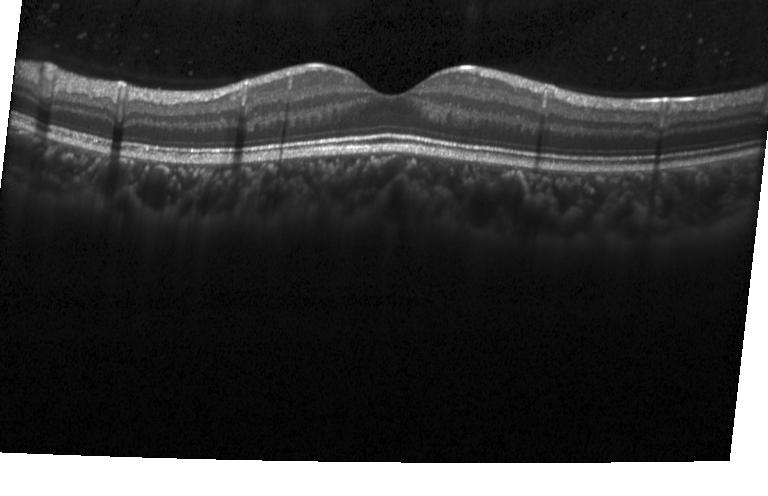

This B-scan demonstrates no choroidal neovascularization, diabetic macular edema, or drusen.